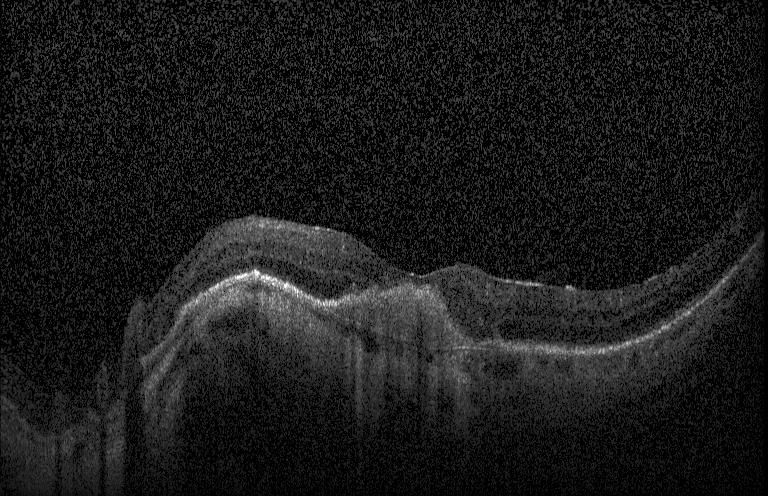 Optical coherence tomography B-scan.
Dx: a choroidal neovascular membrane.